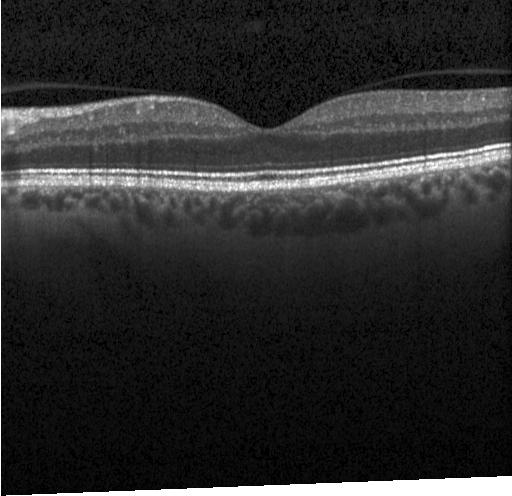 Spectral-domain OCT B-scan: neither CNV, DME, nor drusen.